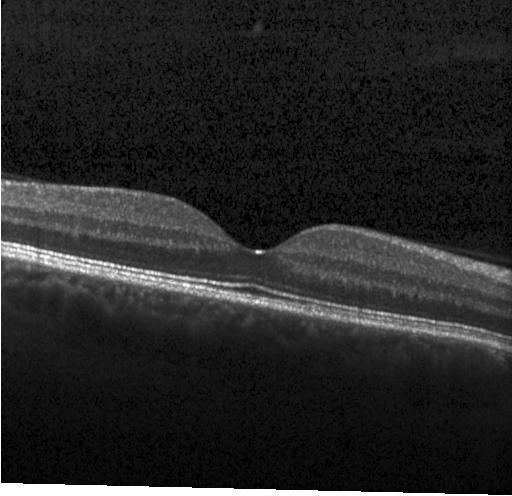 OCT line scan
OCT finding: neither choroidal neovascularization, diabetic macular edema, nor drusen.